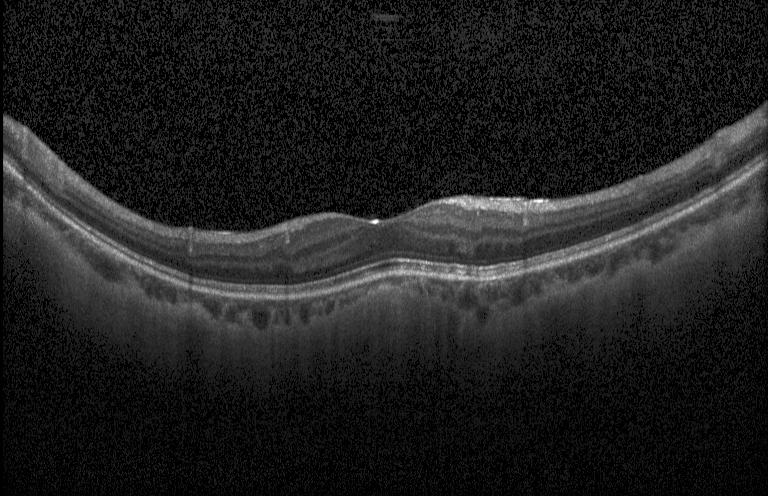
Heidelberg Spectralis OCT system; spectral-domain optical coherence tomography; OCT B-scan — This B-scan demonstrates neither choroidal neovascularization, diabetic macular edema, nor drusen.